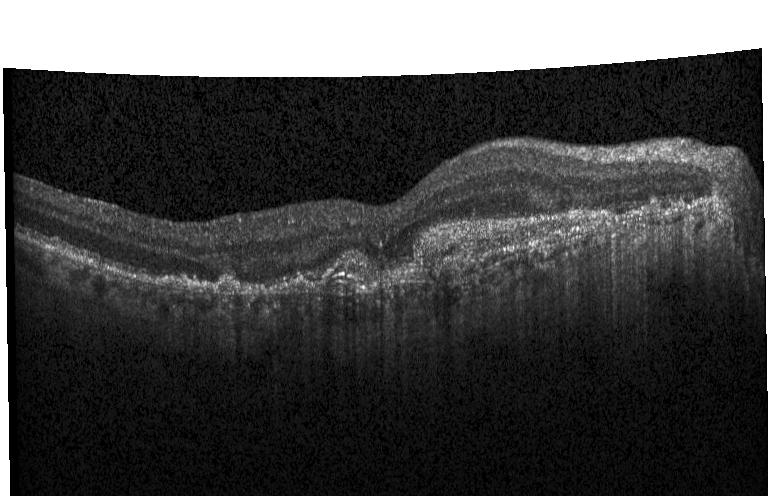

Finding: a choroidal neovascular membrane.